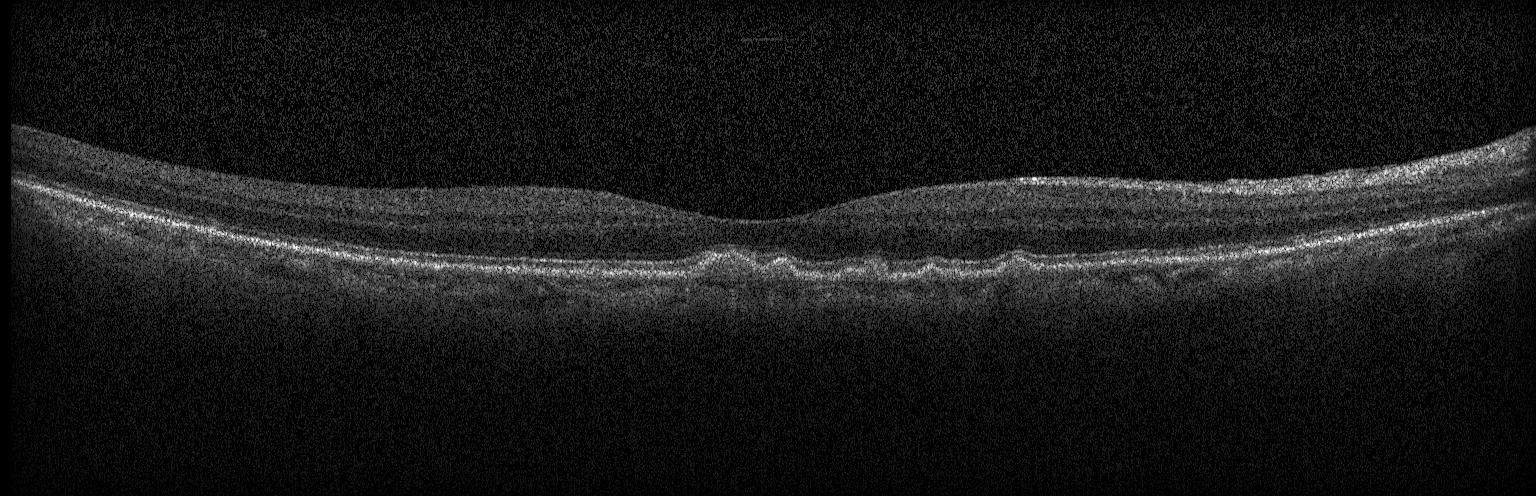
Impression: drusen.